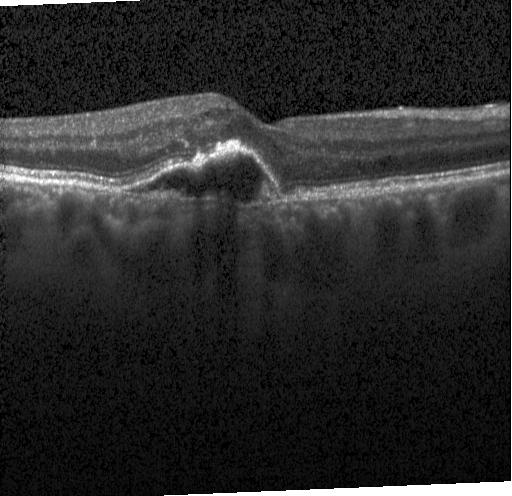 OCT scan showing a choroidal neovascular membrane.